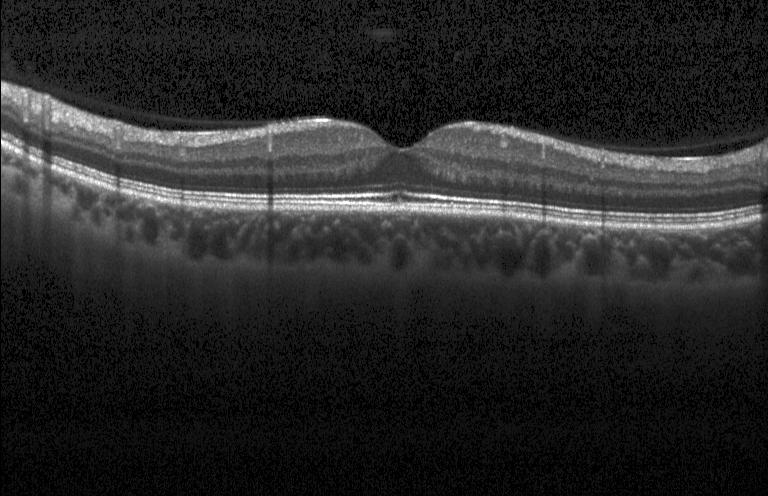

Finding: neither choroidal neovascularization, diabetic macular edema, nor drusen.